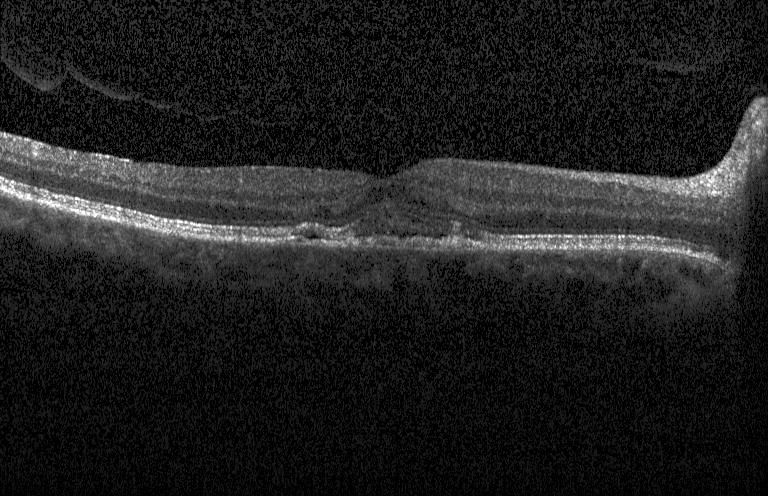 Impression: a choroidal neovascular membrane.